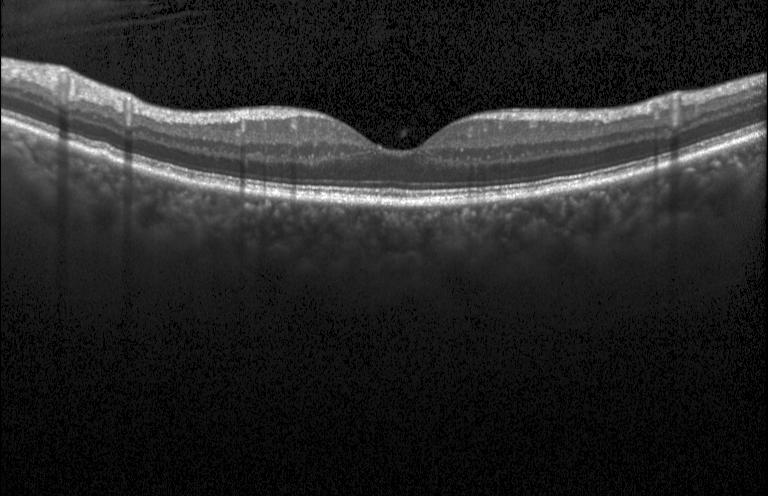

Retinal OCT cross-section. The scan shows no choroidal neovascularization, no diabetic macular edema, and no drusen.